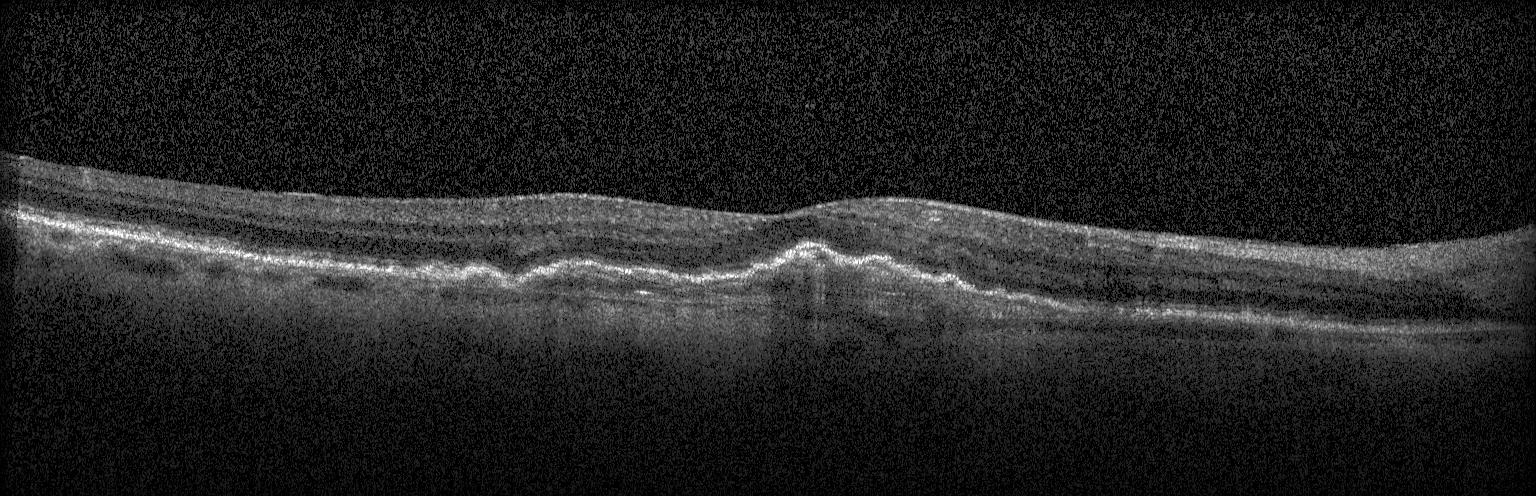
Macular scan; spectral-domain OCT; OCT line scan
Impression: CNV.